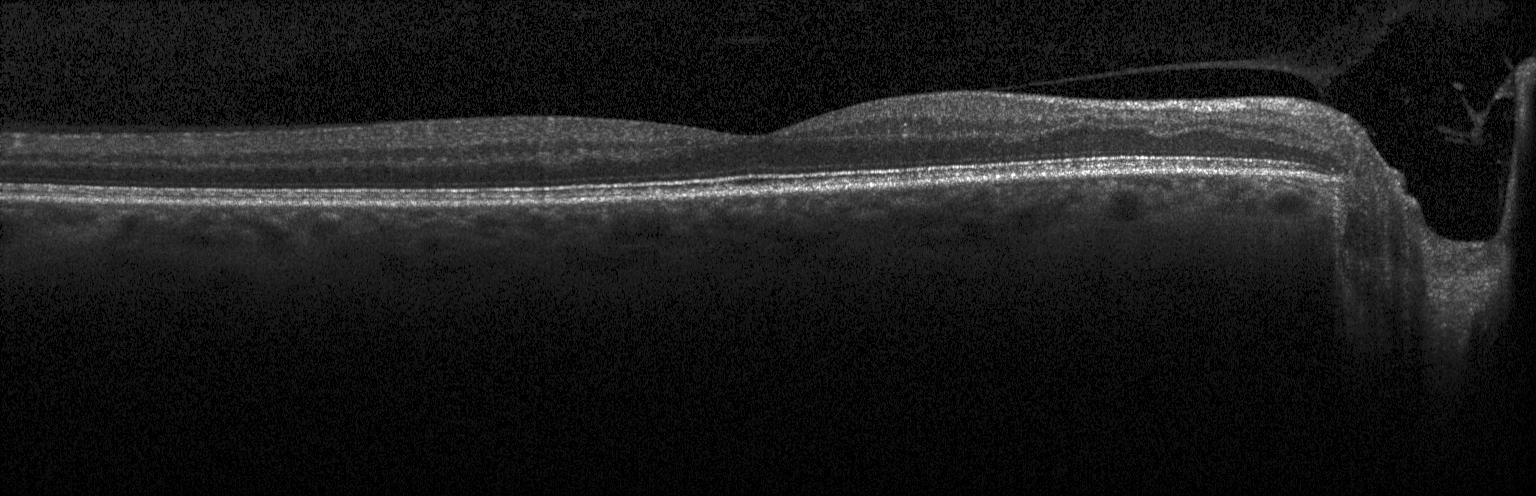 OCT line scan. Diagnosis: no CNV, no DME, and no drusen.